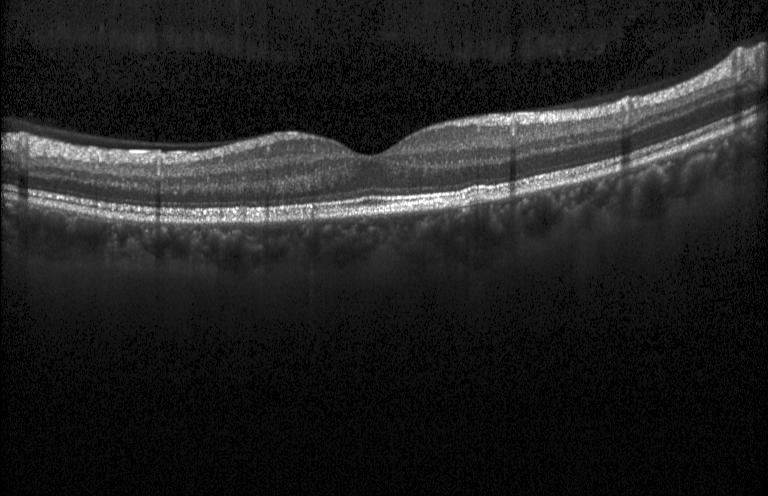 OCT B-scan showing sub-RPE drusenoid deposits.